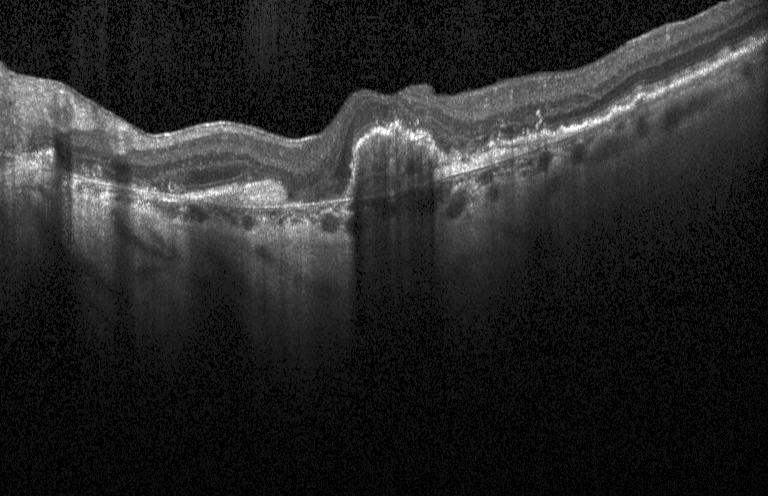

SD-OCT; Heidelberg Spectralis OCT system; optical coherence tomography scan.
Impression: a choroidal neovascular membrane.